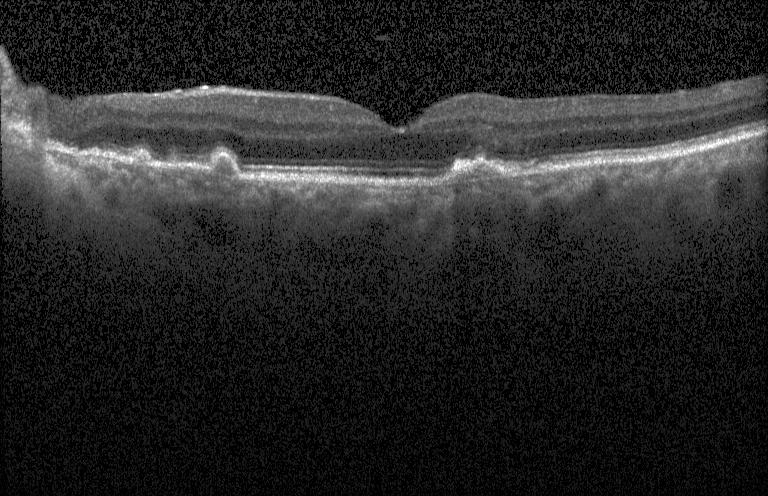

OCT line scan
The scan shows sub-RPE drusenoid deposits.